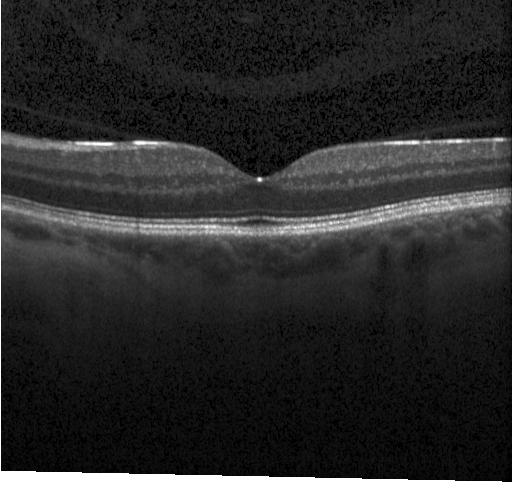 Optical coherence tomography scan — This B-scan demonstrates no evidence of choroidal neovascularization, diabetic macular edema, or drusen.